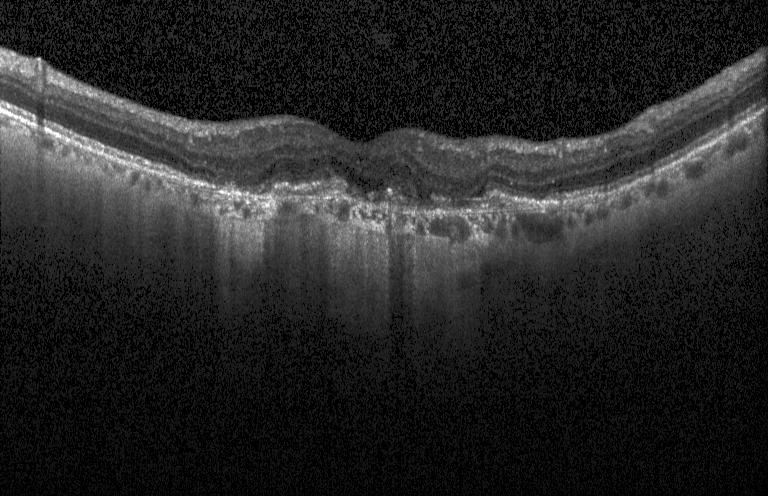 Spectral-domain OCT; optical coherence tomography B-scan.
Finding: choroidal neovascularization (CNV).